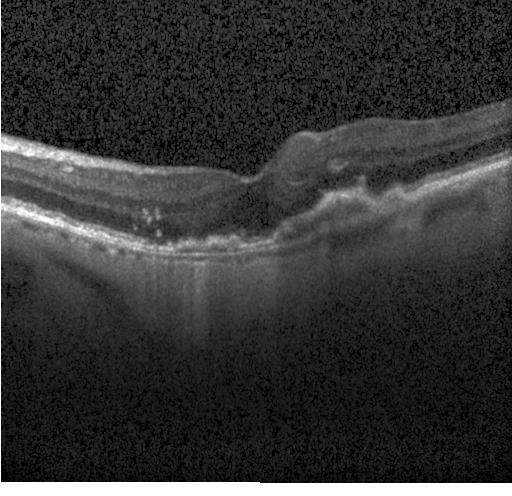

Spectral-domain OCT B-scan: CNV.